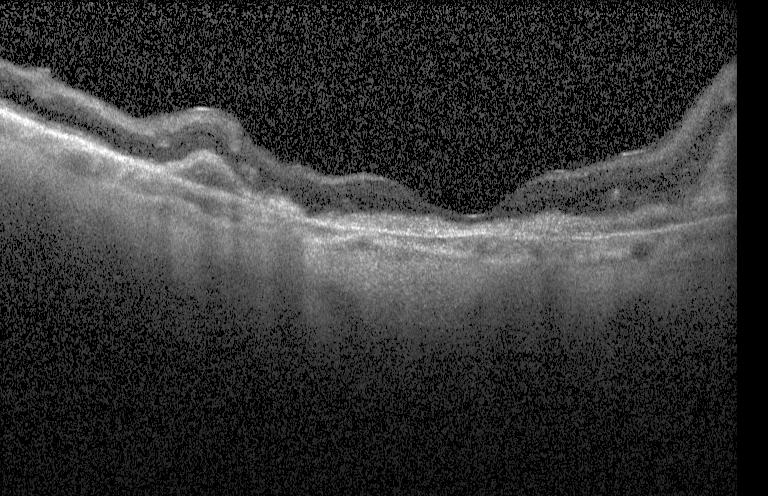 Fovea-centered; OCT B-scan
Impression: a choroidal neovascular membrane.